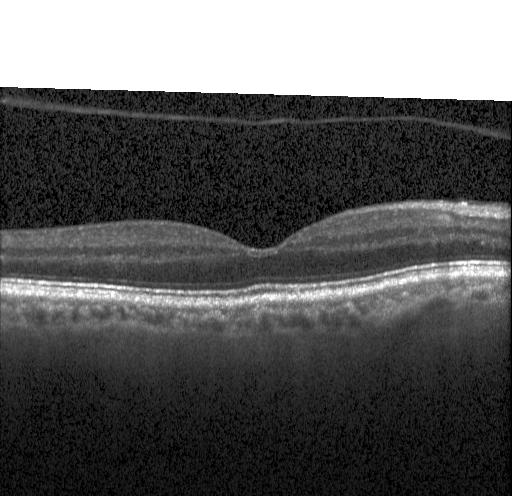
Diagnosis: no choroidal neovascularization, diabetic macular edema, or drusen.